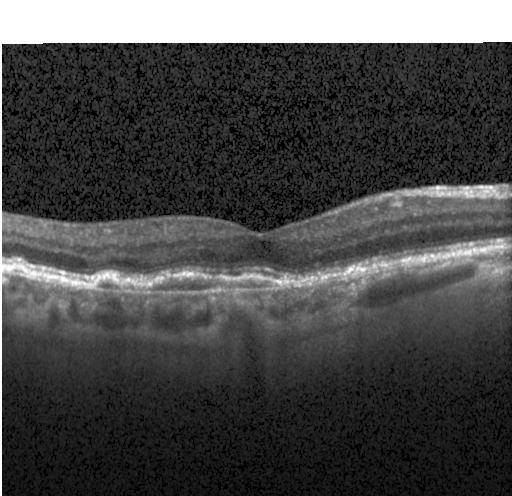
Heidelberg Spectralis, through the macula, OCT line scan, spectral-domain optical coherence tomography.
This B-scan demonstrates a choroidal neovascular membrane.